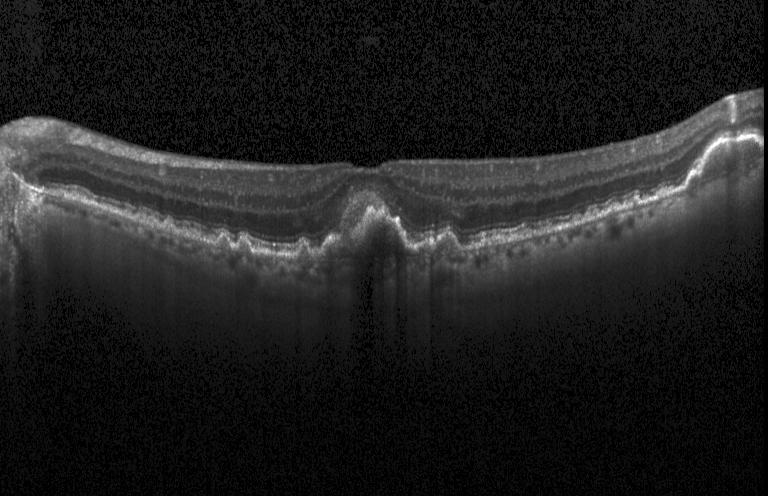

Optical coherence tomography B-scan
This B-scan demonstrates a choroidal neovascular membrane.